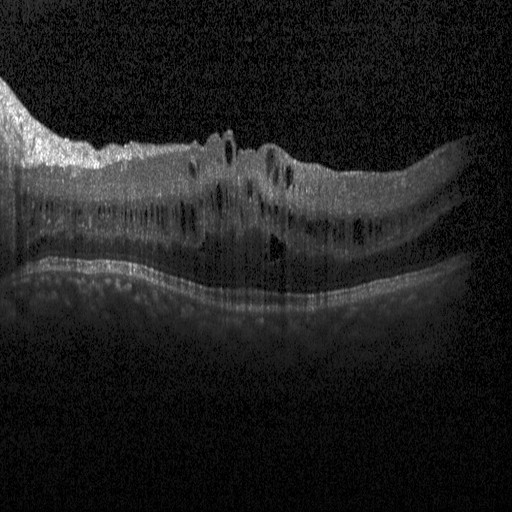 OCT B-scan showing DME.